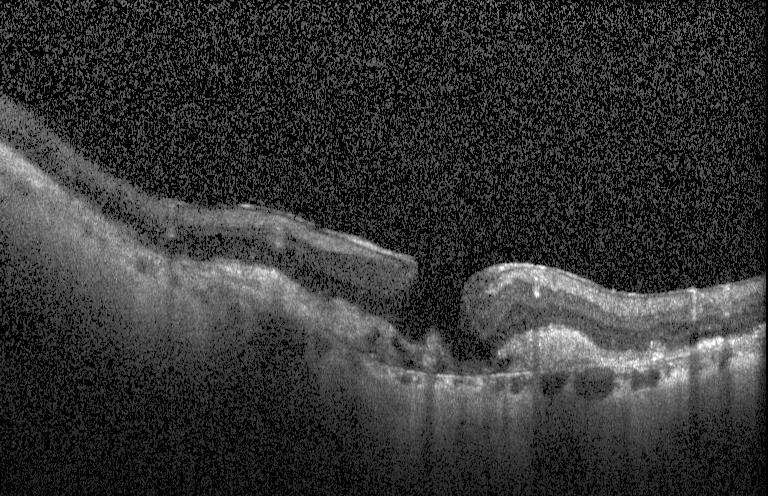

Optical coherence tomography scan — A choroidal neovascular membrane.